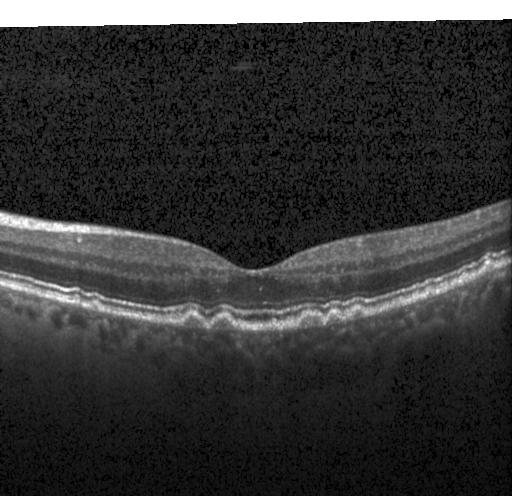

SD-OCT, through the macula, OCT line scan, Heidelberg Spectralis — OCT finding: multiple drusen.